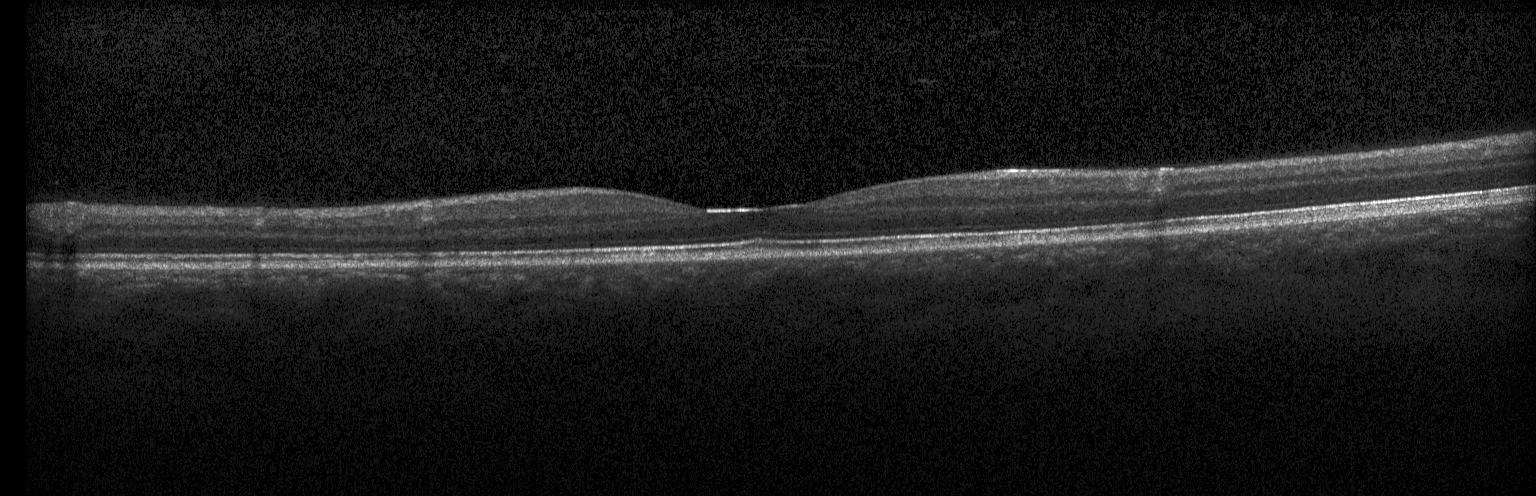

The scan shows no choroidal neovascularization, diabetic macular edema, or drusen.